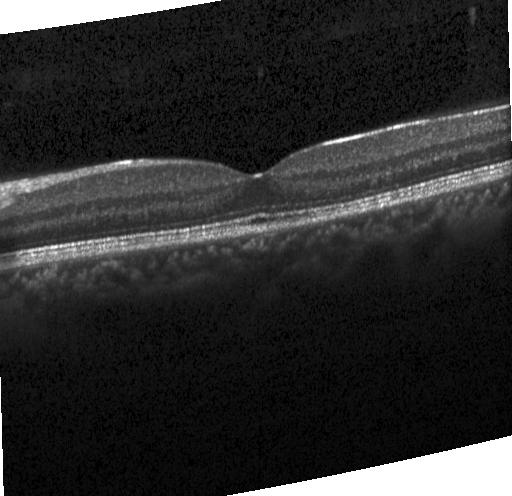
Retinal OCT cross-section; SD-OCT.
OCT finding: no choroidal neovascularization, diabetic macular edema, or drusen.